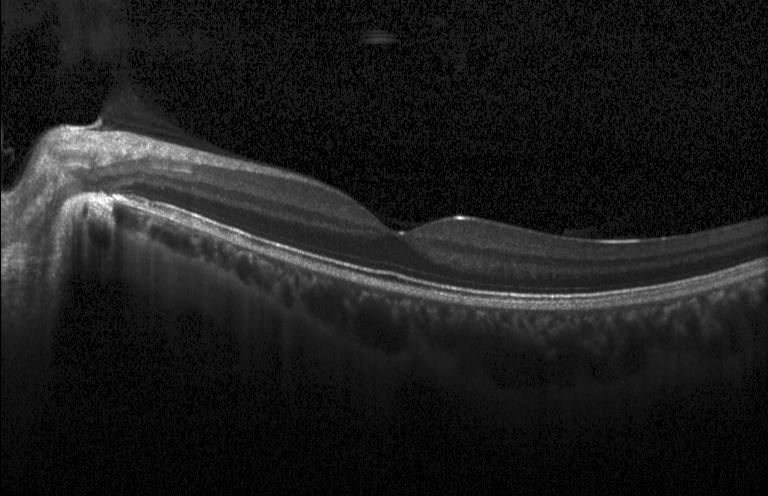
Impression: no choroidal neovascularization, diabetic macular edema, or drusen.